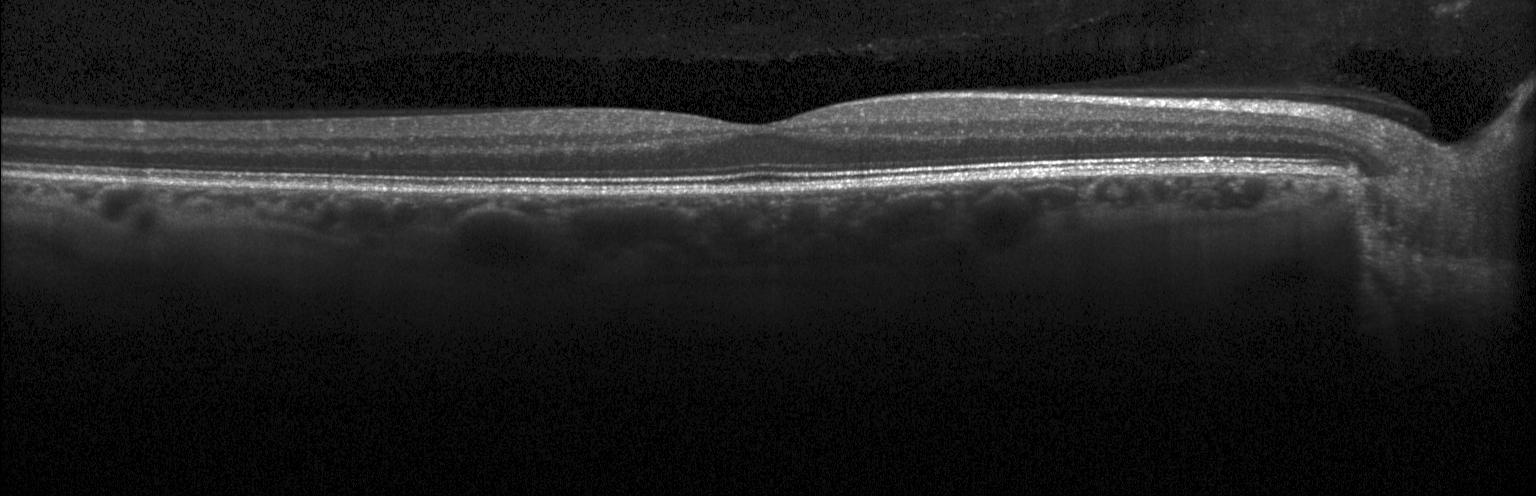 Retinal OCT B-scan; Heidelberg Spectralis OCT system; spectral-domain optical coherence tomography
OCT finding: no evidence of choroidal neovascularization, diabetic macular edema, or drusen.